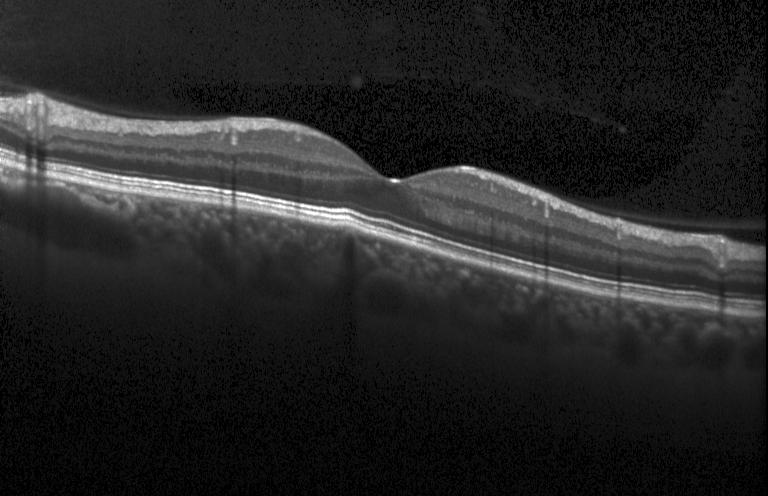

Acquired on a Heidelberg Spectralis, spectral-domain optical coherence tomography, fovea-centered, OCT B-scan
This B-scan demonstrates no CNV, DME, or drusen.